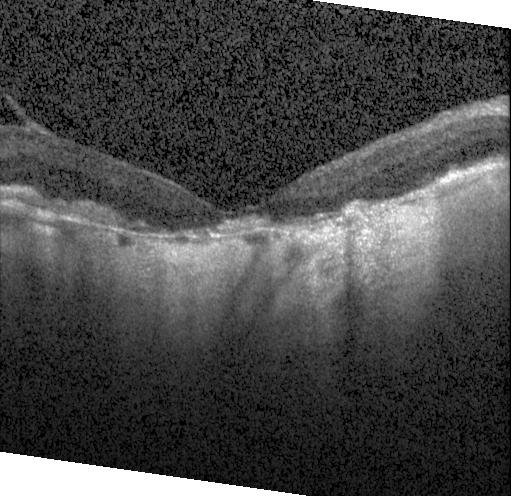

Optical coherence tomography scan · SD-OCT.
Assessment: choroidal neovascularization (CNV).